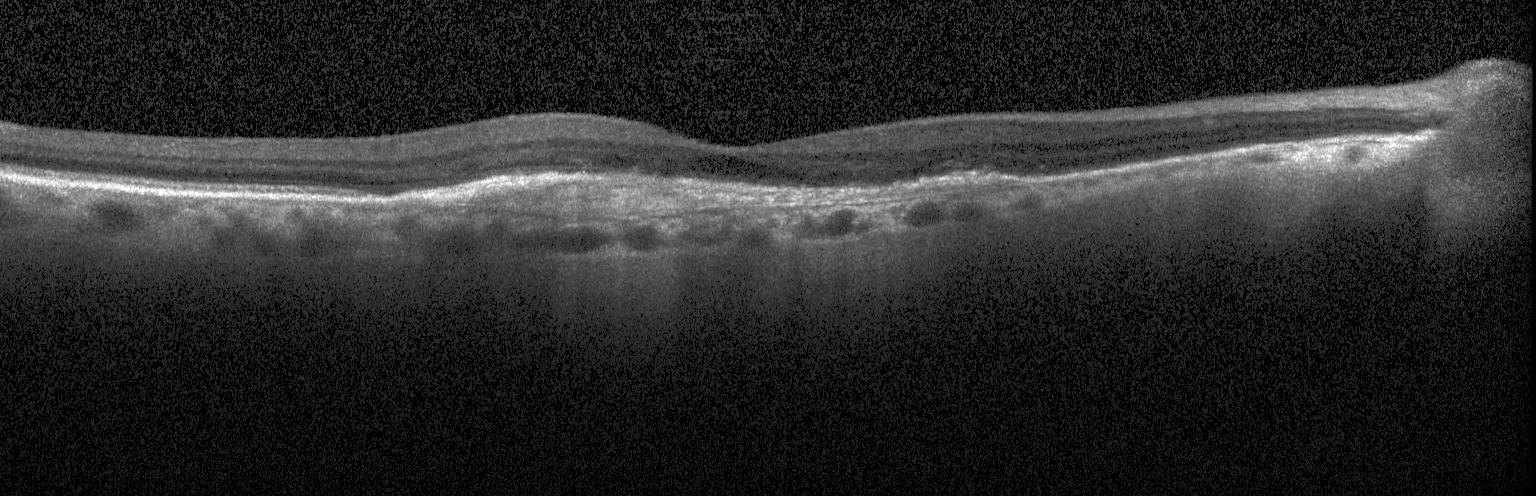 Macular OCT: a choroidal neovascular membrane.